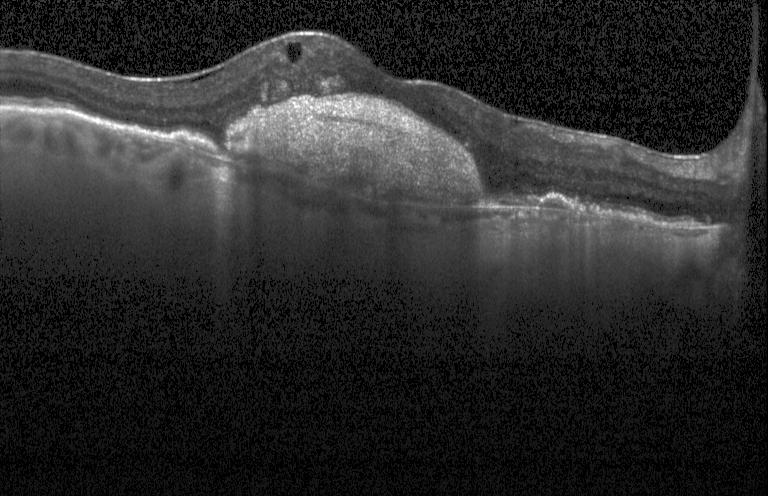 Impression: choroidal neovascularization (CNV).